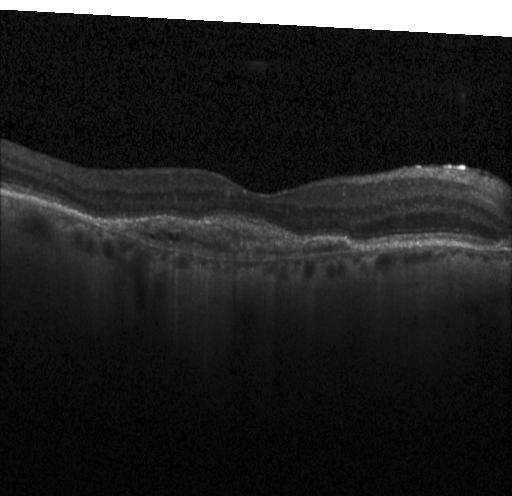 Acquired on a Heidelberg Spectralis. Macular scan. Spectral-domain optical coherence tomography. OCT B-scan. Impression: a choroidal neovascular membrane.